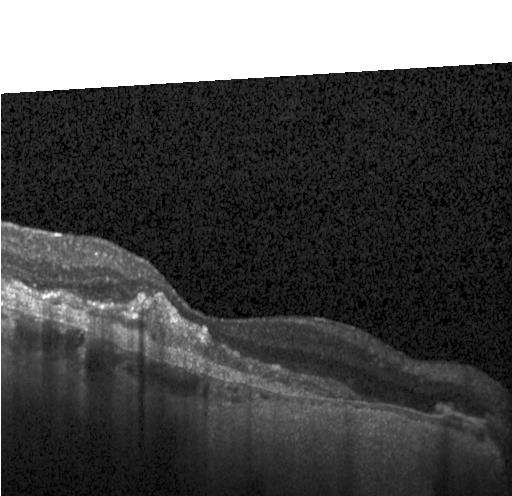 Retinal OCT cross-section. Macular scan. Heidelberg Spectralis OCT system. Spectral-domain optical coherence tomography. The scan shows a choroidal neovascular membrane.